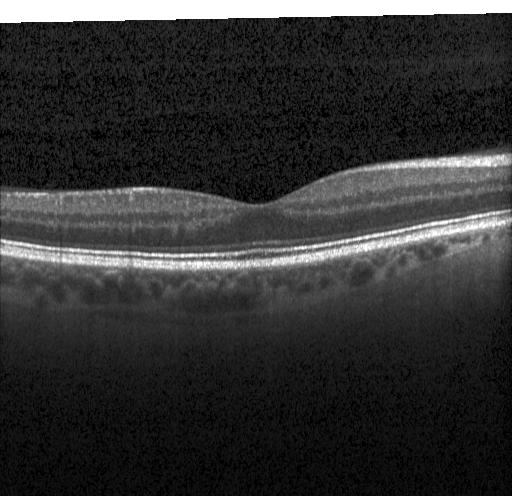 Fovea-centered; optical coherence tomography scan. The scan shows no choroidal neovascularization, diabetic macular edema, or drusen.